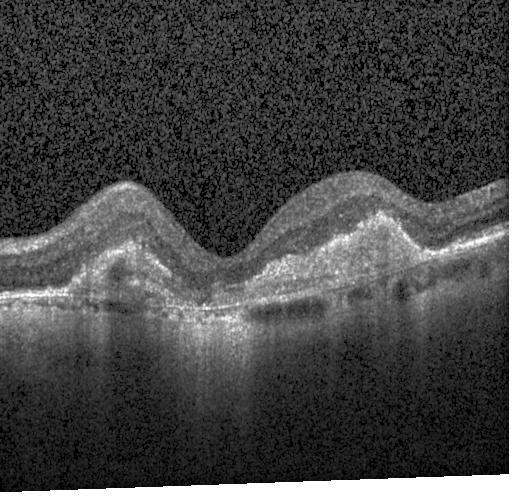
Optical coherence tomography B-scan
This B-scan demonstrates choroidal neovascularization.